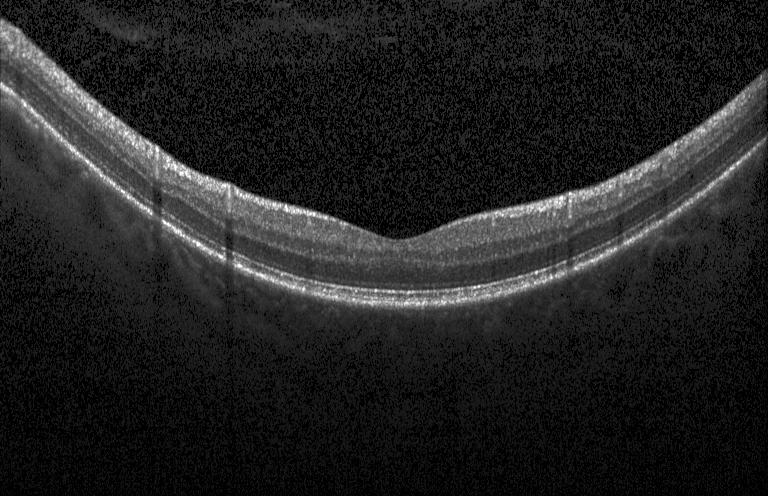 OCT B-scan · spectral-domain optical coherence tomography. Impression: no evidence of choroidal neovascularization, diabetic macular edema, or drusen.